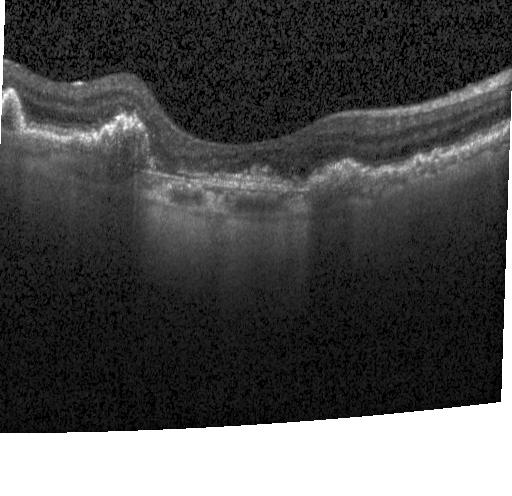 OCT B-scan, macular scan, instrument: Heidelberg Spectralis.
Assessment: choroidal neovascularization (CNV).